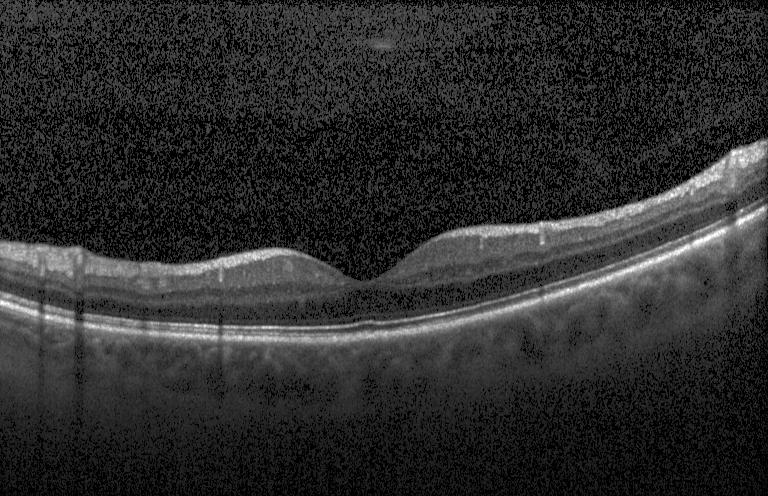

Retinal OCT B-scan, fovea-centered
Macular OCT: no choroidal neovascularization, diabetic macular edema, or drusen.